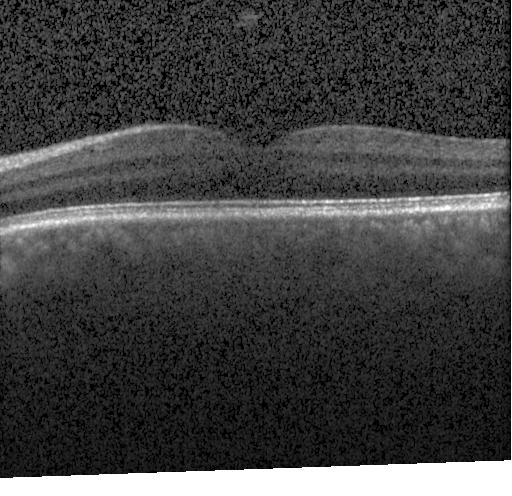 Retinal OCT B-scan.
OCT finding: neither choroidal neovascularization, diabetic macular edema, nor drusen.